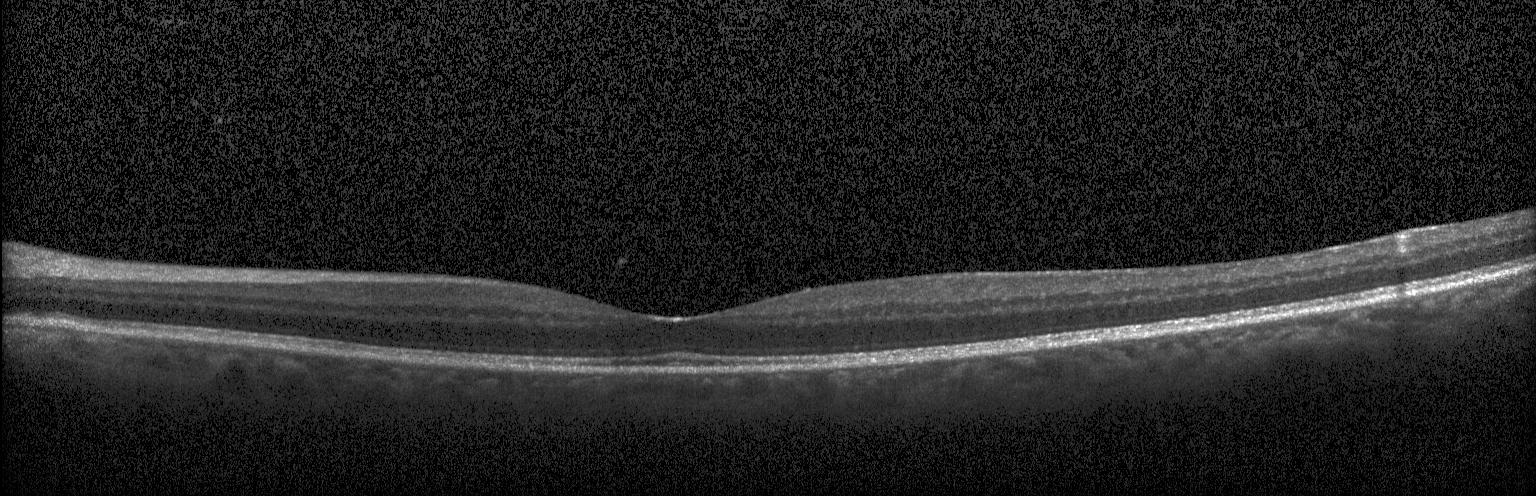 Instrument: Heidelberg Spectralis. OCT B-scan. SD-OCT. No evidence of choroidal neovascularization, diabetic macular edema, or drusen.